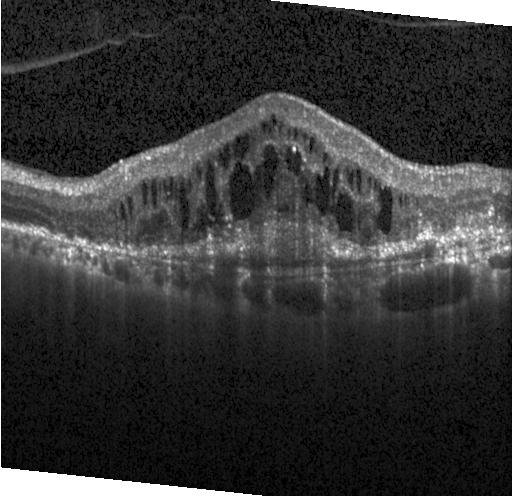

Acquired on a Heidelberg Spectralis. Through the macula. Optical coherence tomography B-scan
Assessment: a choroidal neovascular membrane.